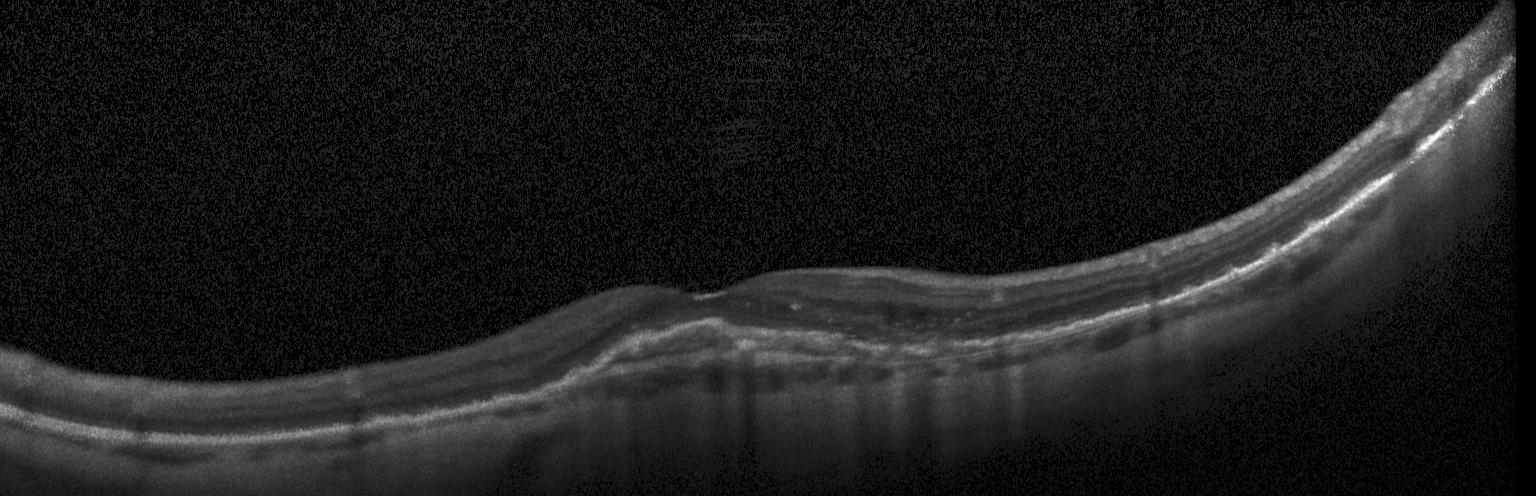

Finding: a choroidal neovascular membrane.